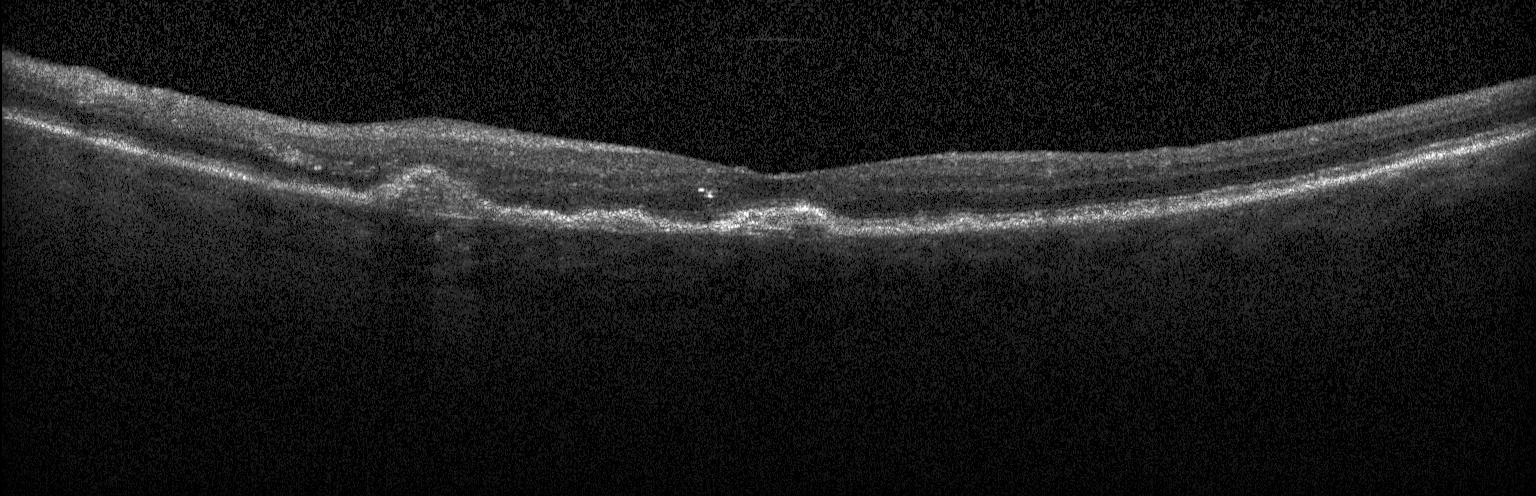 OCT B-scan showing choroidal neovascularization (CNV).